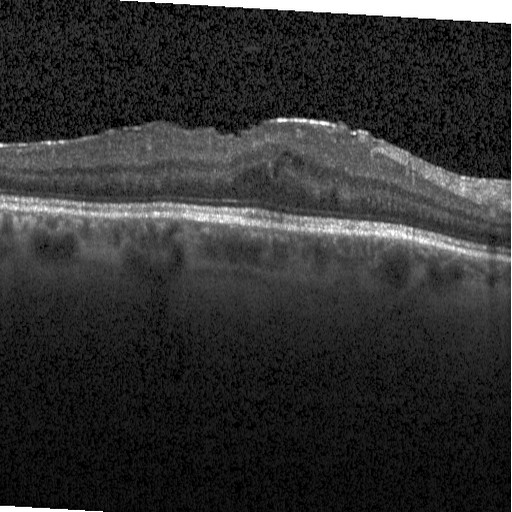

Spectral-domain OCT, optical coherence tomography B-scan, fovea-centered — This B-scan demonstrates DME.